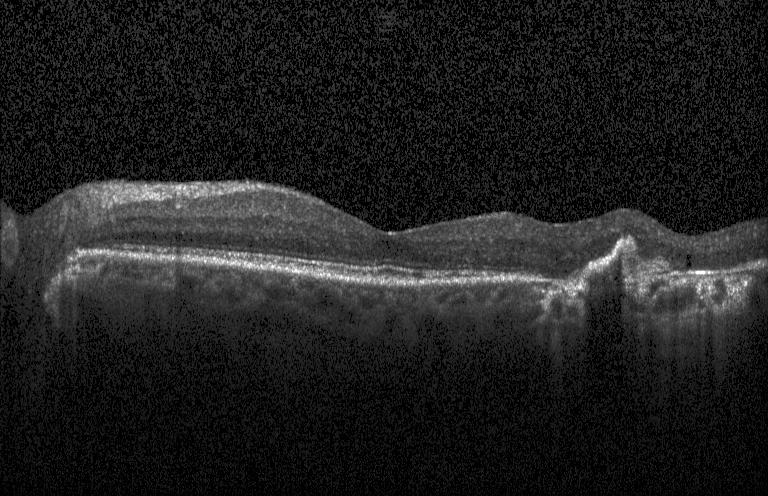

Optical coherence tomography B-scan · fovea-centered. OCT finding: choroidal neovascularization.